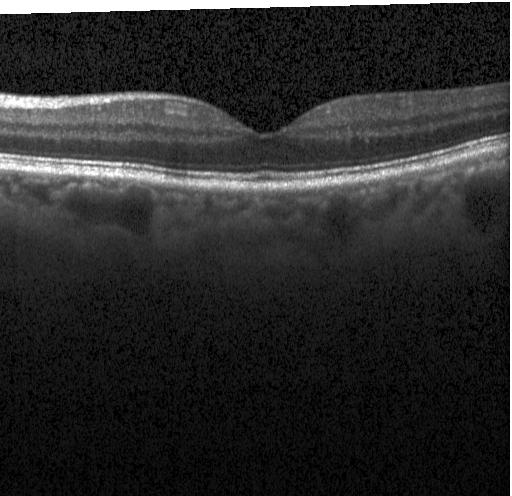 OCT line scan
No choroidal neovascularization, diabetic macular edema, or drusen.